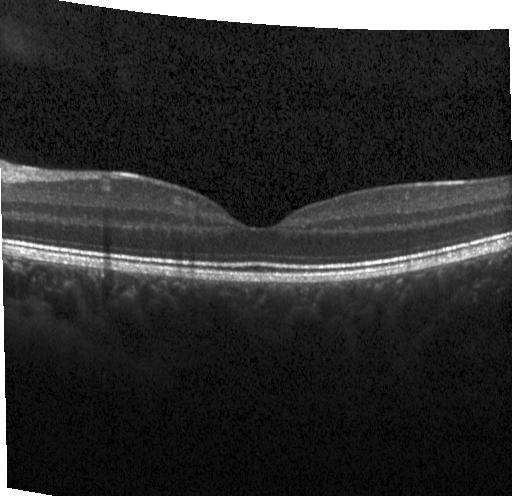 Retinal OCT cross-section
Impression: neither choroidal neovascularization, diabetic macular edema, nor drusen.